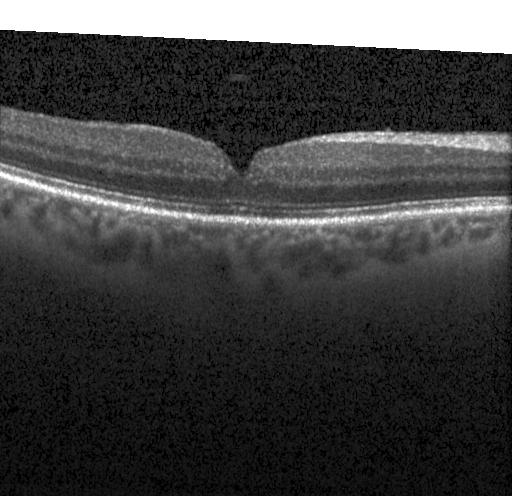
Optical coherence tomography scan · spectral-domain OCT · Heidelberg Spectralis OCT system · macular scan
Diagnosis: no CNV, DME, or drusen.